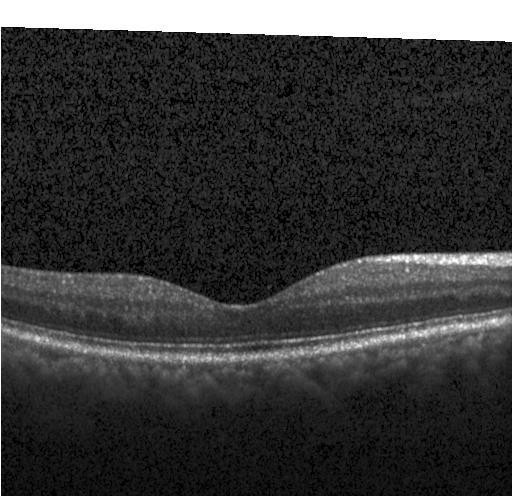
OCT B-scan showing no evidence of choroidal neovascularization, diabetic macular edema, or drusen.